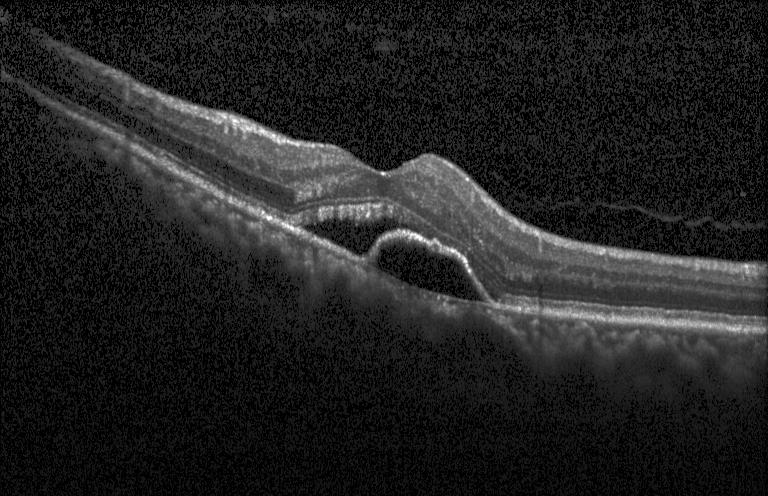 Spectral-domain OCT B-scan: a choroidal neovascular membrane.